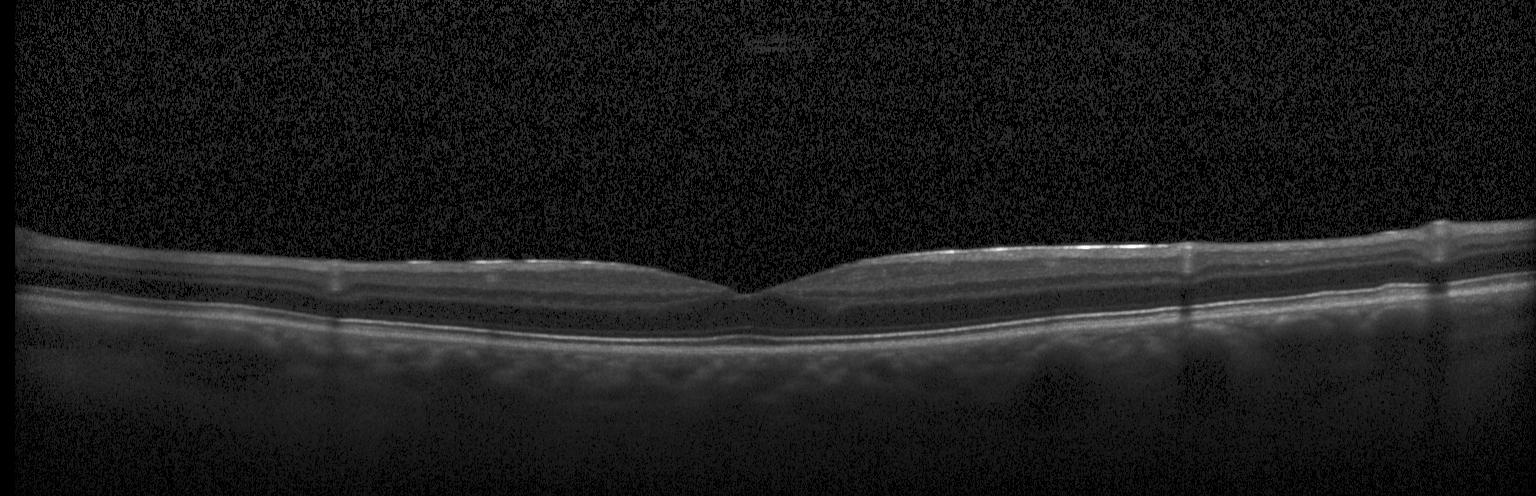 Optical coherence tomography scan. Horizontal scan through the fovea — Diagnosis: no choroidal neovascularization, no diabetic macular edema, and no drusen.